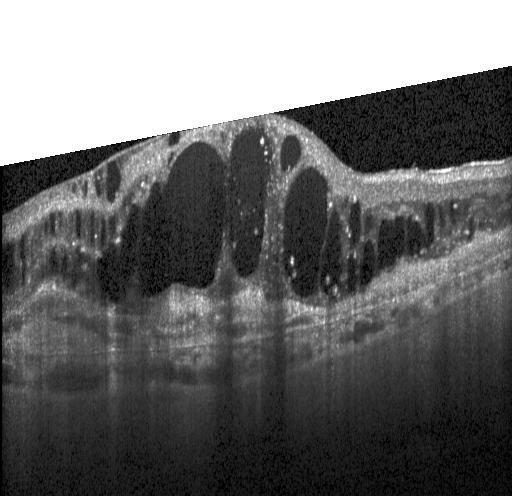 Retinal OCT B-scan, spectral-domain OCT.
A choroidal neovascular membrane.